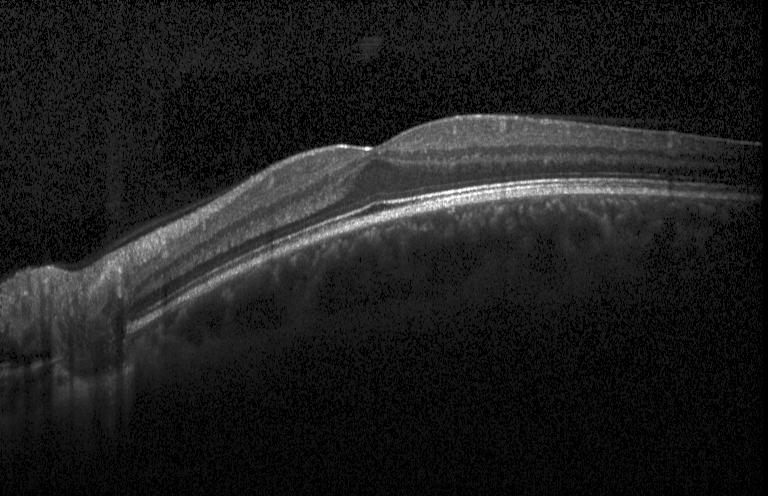
Macular OCT demonstrating neither CNV, DME, nor drusen.